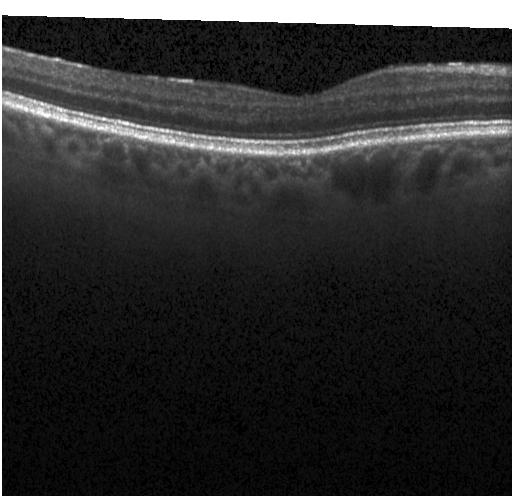 Assessment: no evidence of choroidal neovascularization, diabetic macular edema, or drusen.